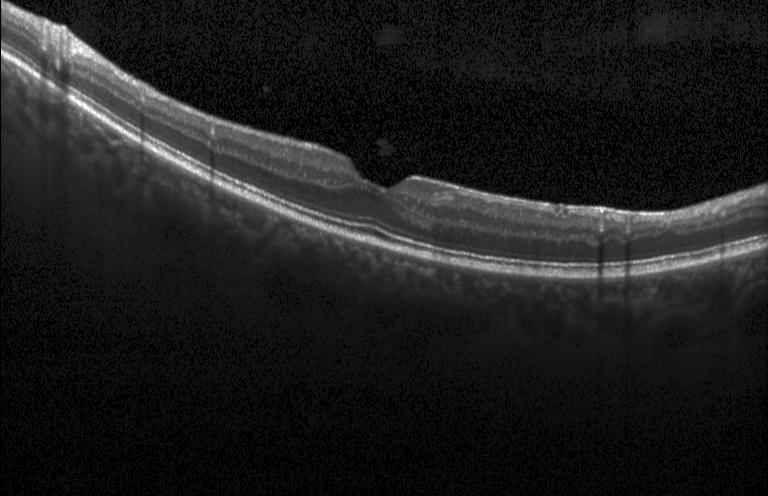 OCT finding: no choroidal neovascularization, diabetic macular edema, or drusen.